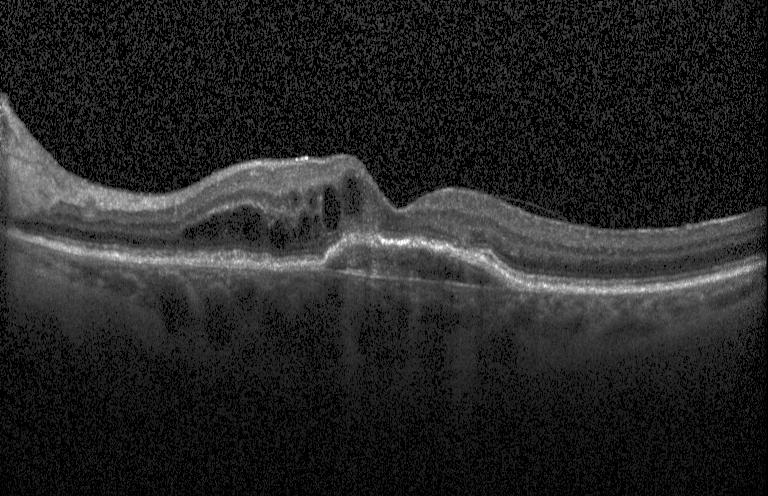
OCT scan showing a choroidal neovascular membrane.